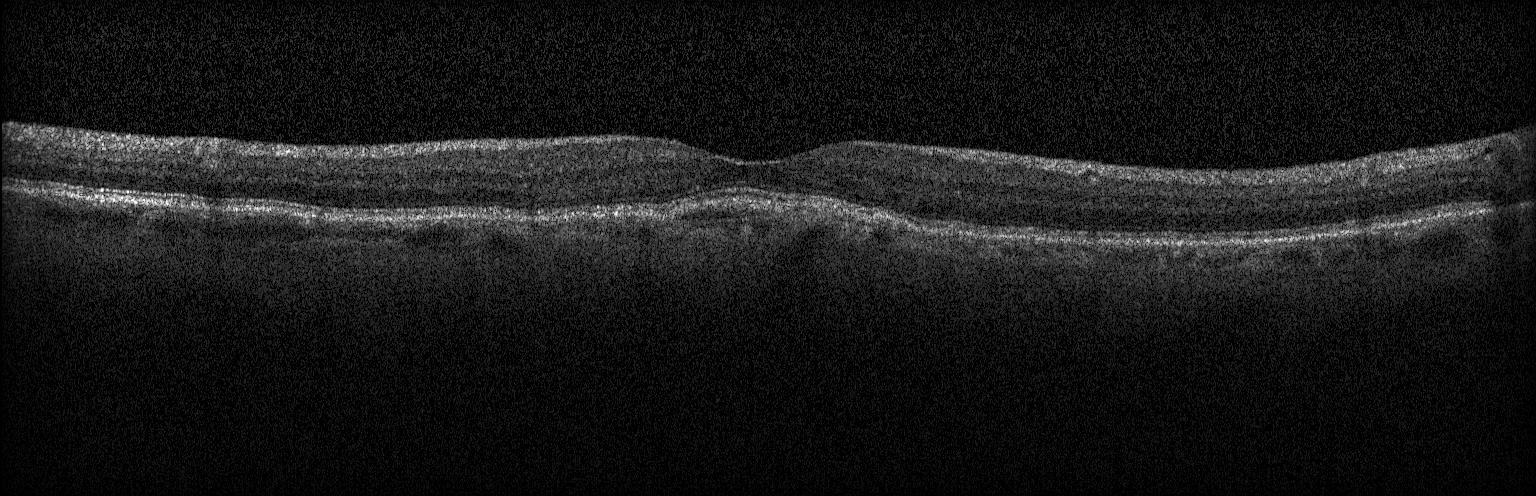

Optical coherence tomography B-scan. SD-OCT.
Assessment: choroidal neovascularization.